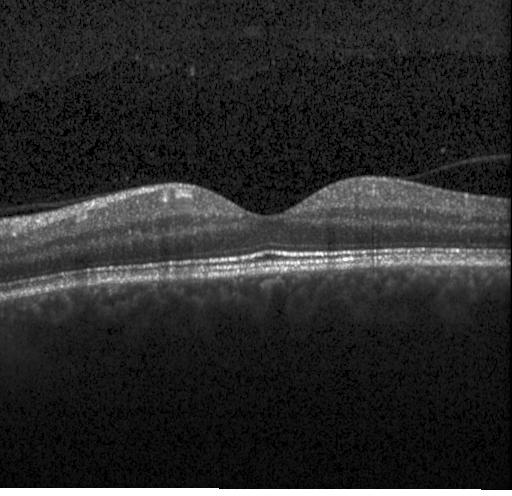
SD-OCT; OCT B-scan; macular scan; acquired on a Heidelberg Spectralis
Impression: no CNV, DME, or drusen.